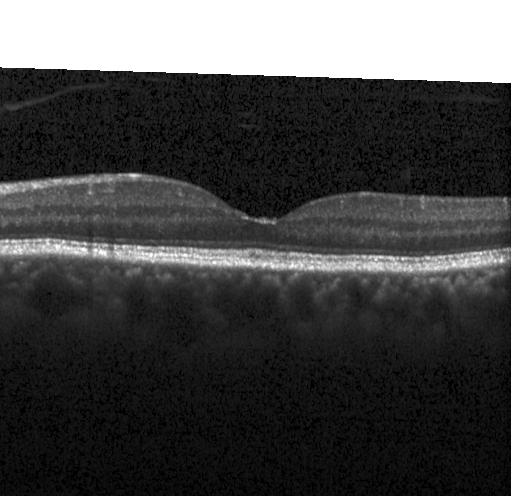
Retinal OCT B-scan. Fovea-centered. Acquired on a Heidelberg Spectralis
Impression: no CNV, DME, or drusen.